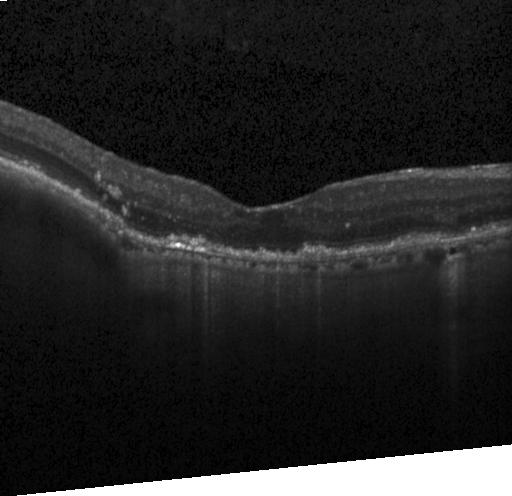

Retinal OCT B-scan, SD-OCT
Finding: CNV.